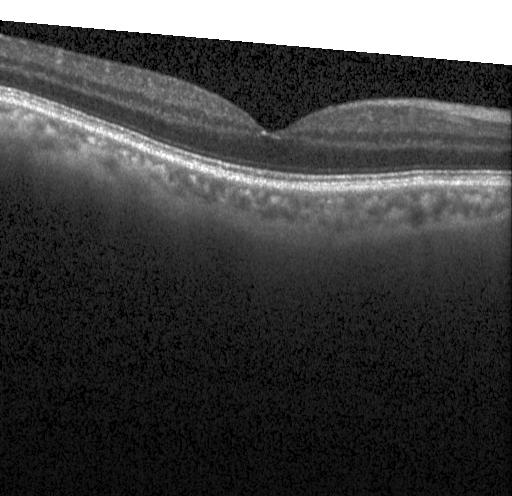 SD-OCT. OCT line scan. Macular scan. Instrument: Heidelberg Spectralis — Finding: no choroidal neovascularization, no diabetic macular edema, and no drusen.